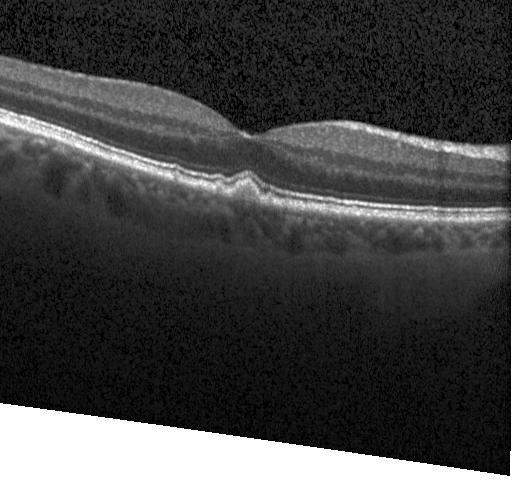
Retinal OCT B-scan. Impression: drusen.